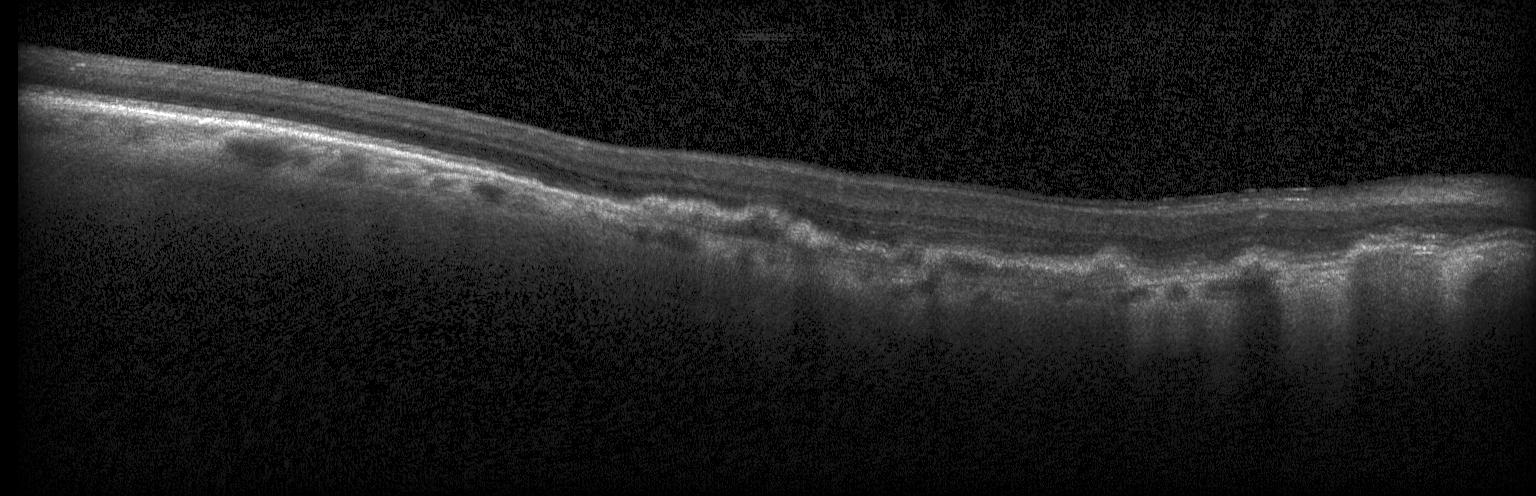
Diagnosis: choroidal neovascularization (CNV).